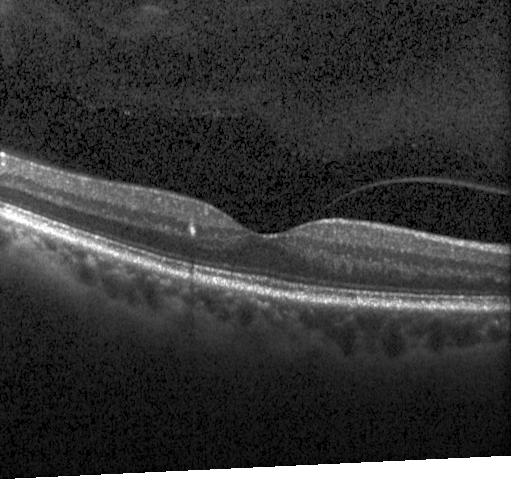
Assessment: no choroidal neovascularization, no diabetic macular edema, and no drusen.